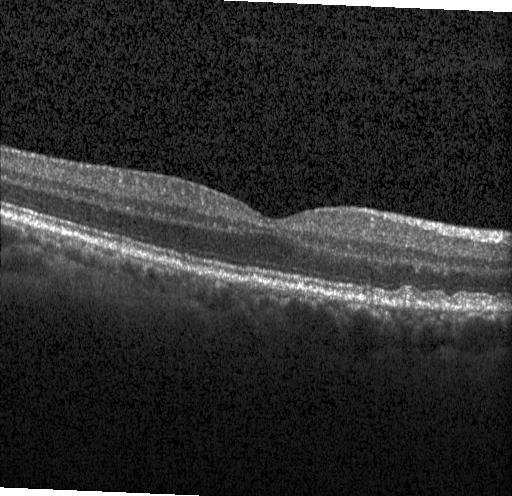 Centered on the fovea. Optical coherence tomography scan. Instrument: Heidelberg Spectralis. The scan shows sub-RPE drusenoid deposits.